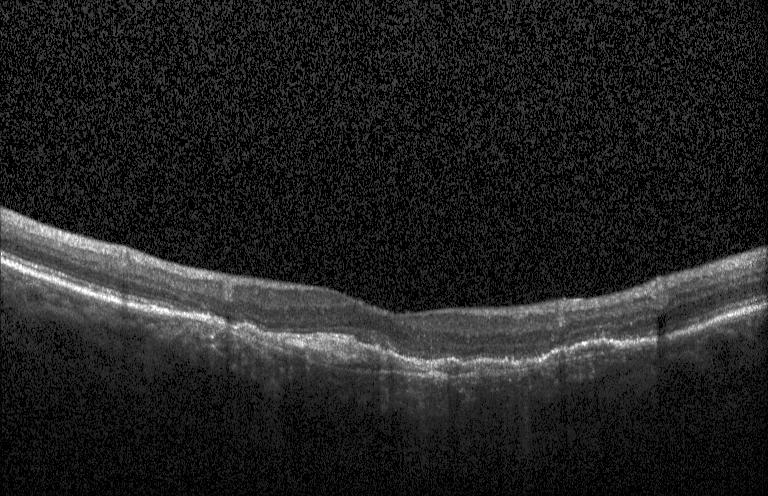

Heidelberg Spectralis OCT system; spectral-domain OCT; through the macula; retinal OCT cross-section
Assessment: CNV.